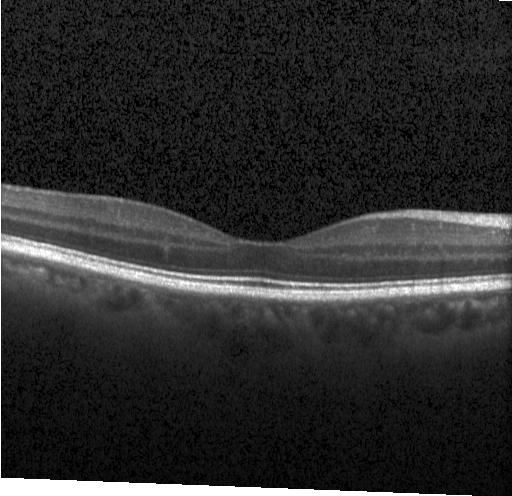

Through the macula, spectral-domain OCT, retinal OCT B-scan.
Finding: no evidence of choroidal neovascularization, diabetic macular edema, or drusen.